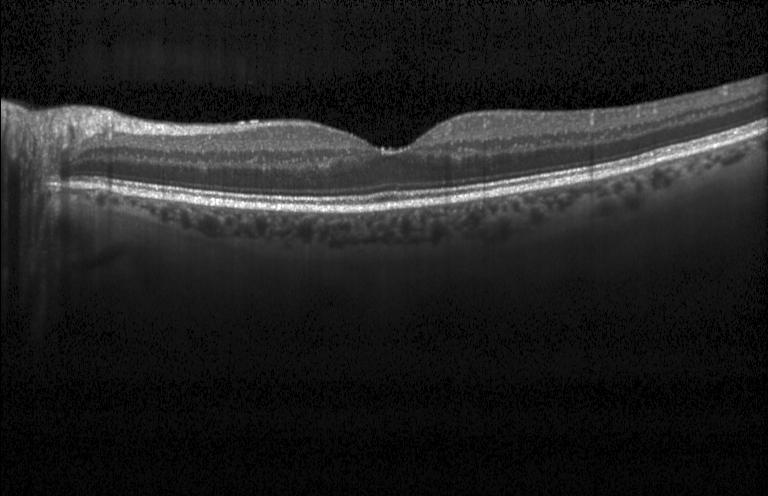 Macular OCT: neither choroidal neovascularization, diabetic macular edema, nor drusen.